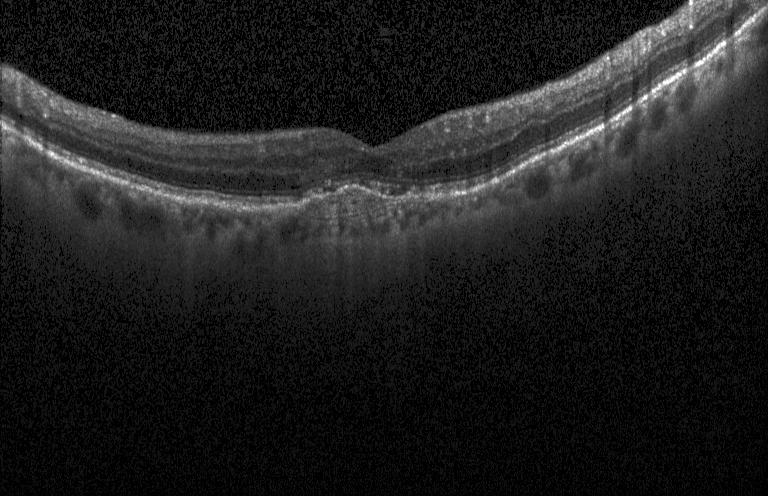

SD-OCT · retinal OCT cross-section. Impression: a choroidal neovascular membrane.